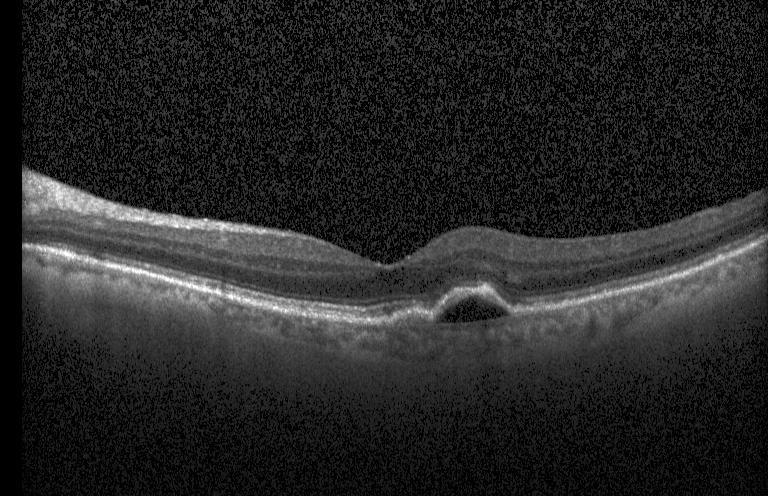
OCT finding: a choroidal neovascular membrane.